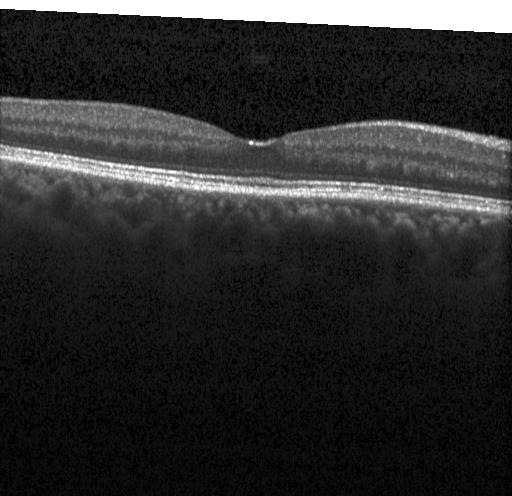 Macular scan, optical coherence tomography B-scan, spectral-domain optical coherence tomography.
Impression: neither choroidal neovascularization, diabetic macular edema, nor drusen.